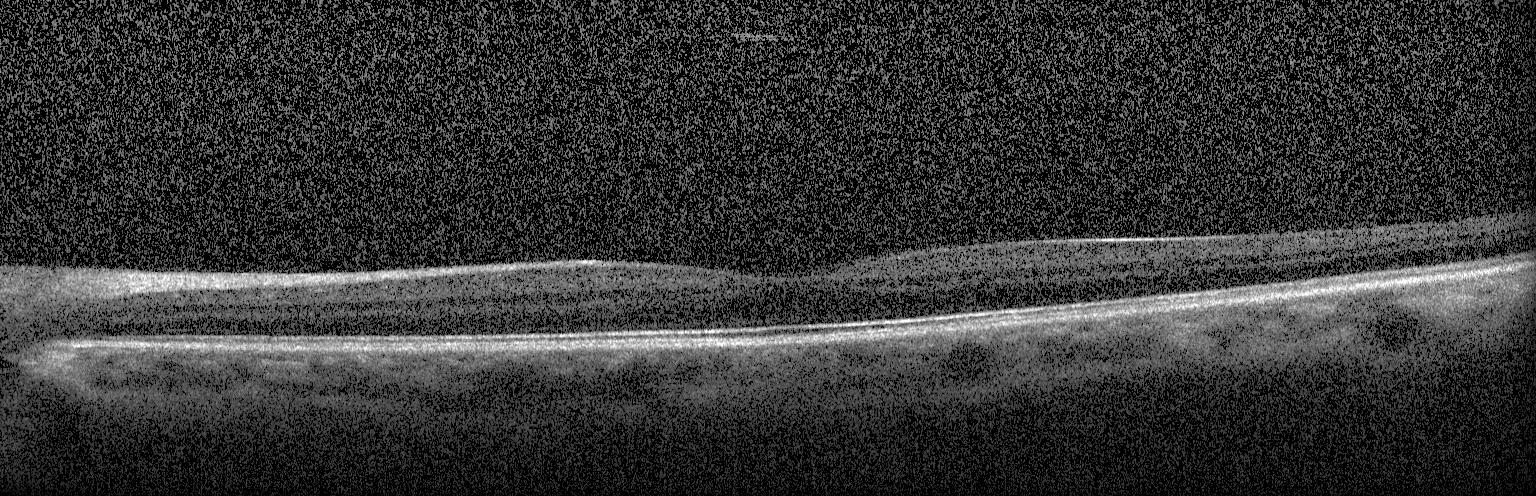

Finding: no choroidal neovascularization, no diabetic macular edema, and no drusen.